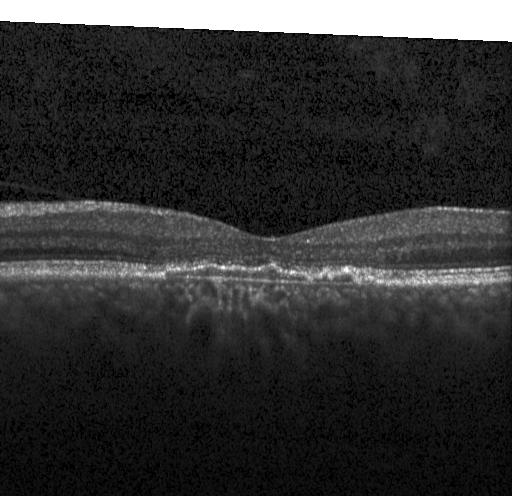 OCT B-scan showing a choroidal neovascular membrane.